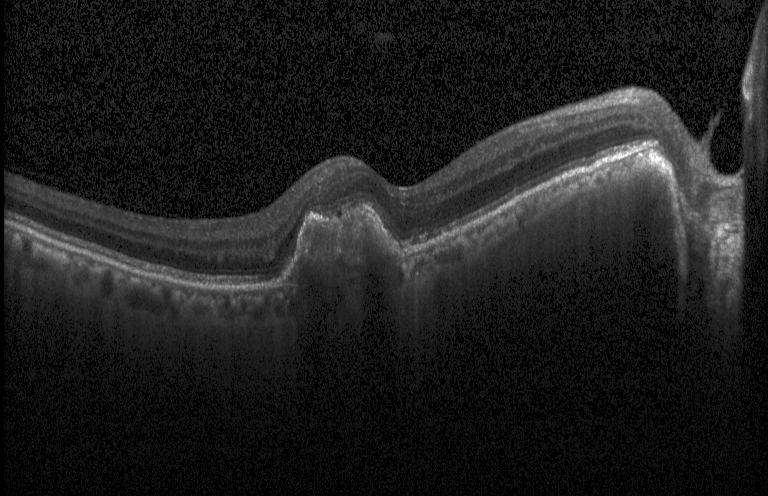

Horizontal scan through the fovea · retinal OCT cross-section. The scan shows CNV.